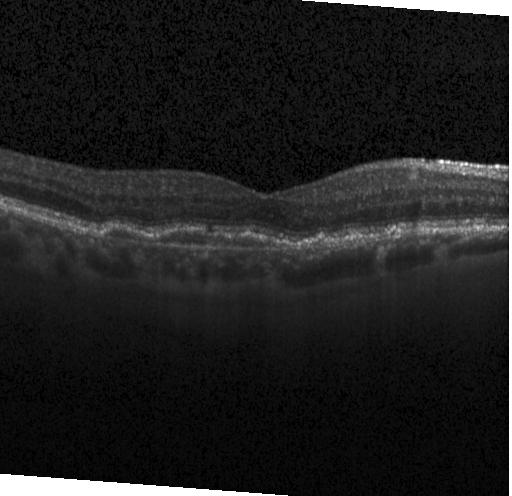 Dx: CNV.